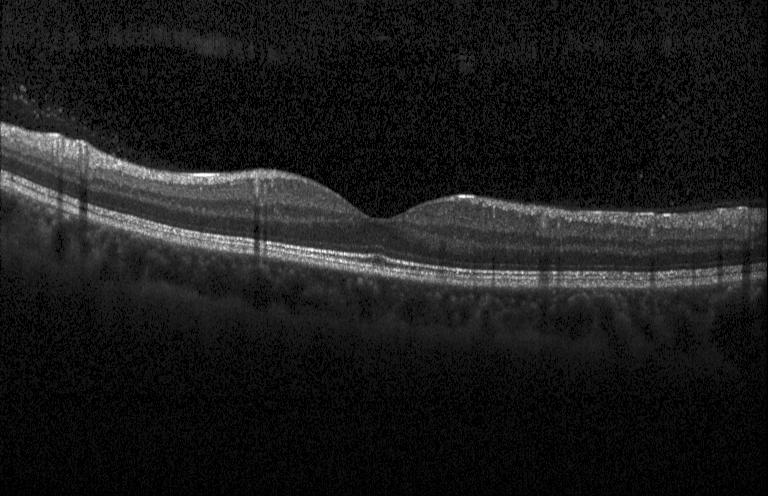

Acquired on a Heidelberg Spectralis, SD-OCT, OCT line scan. Impression: neither choroidal neovascularization, diabetic macular edema, nor drusen.